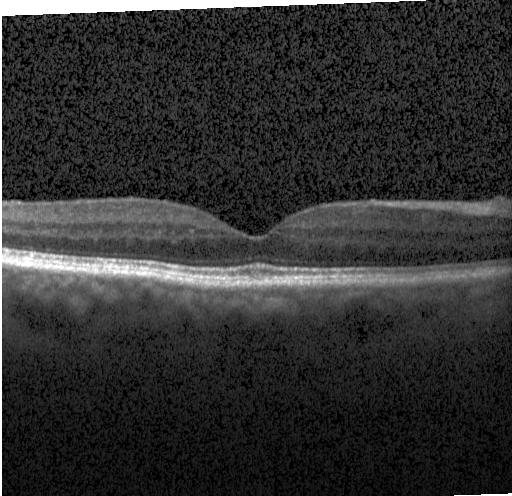

OCT line scan; centered on the fovea
Diagnosis: no evidence of choroidal neovascularization, diabetic macular edema, or drusen.